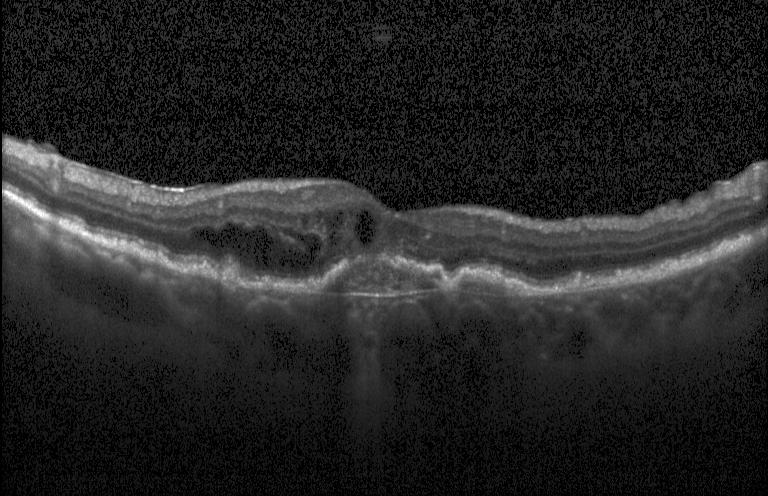 Acquired on a Heidelberg Spectralis · OCT B-scan.
Impression: a choroidal neovascular membrane.